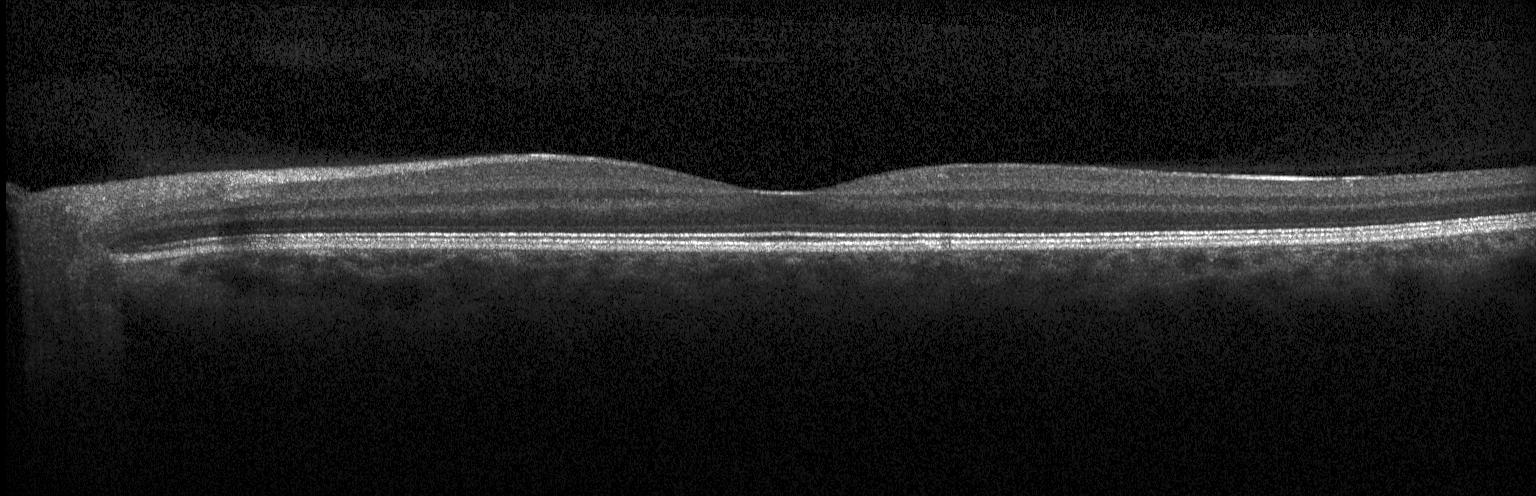

SD-OCT, OCT B-scan, acquired on a Heidelberg Spectralis, fovea-centered. Impression: neither choroidal neovascularization, diabetic macular edema, nor drusen.